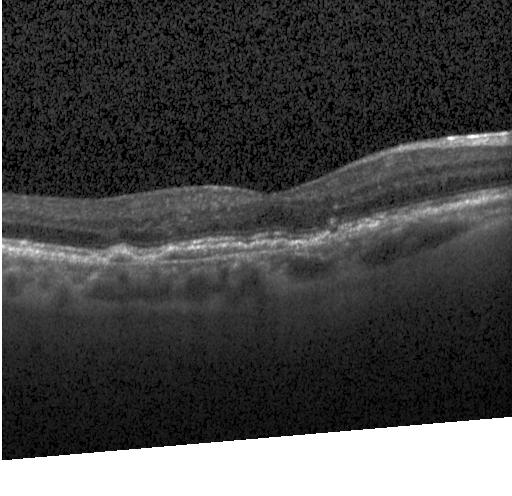
Optical coherence tomography scan. The scan shows a choroidal neovascular membrane.